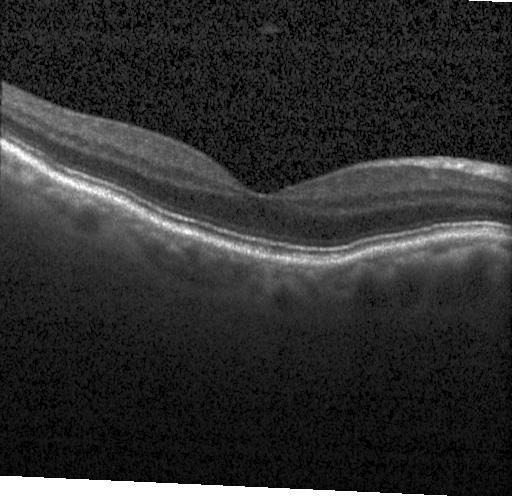

OCT line scan, spectral-domain OCT, macular scan — Finding: no choroidal neovascularization, no diabetic macular edema, and no drusen.